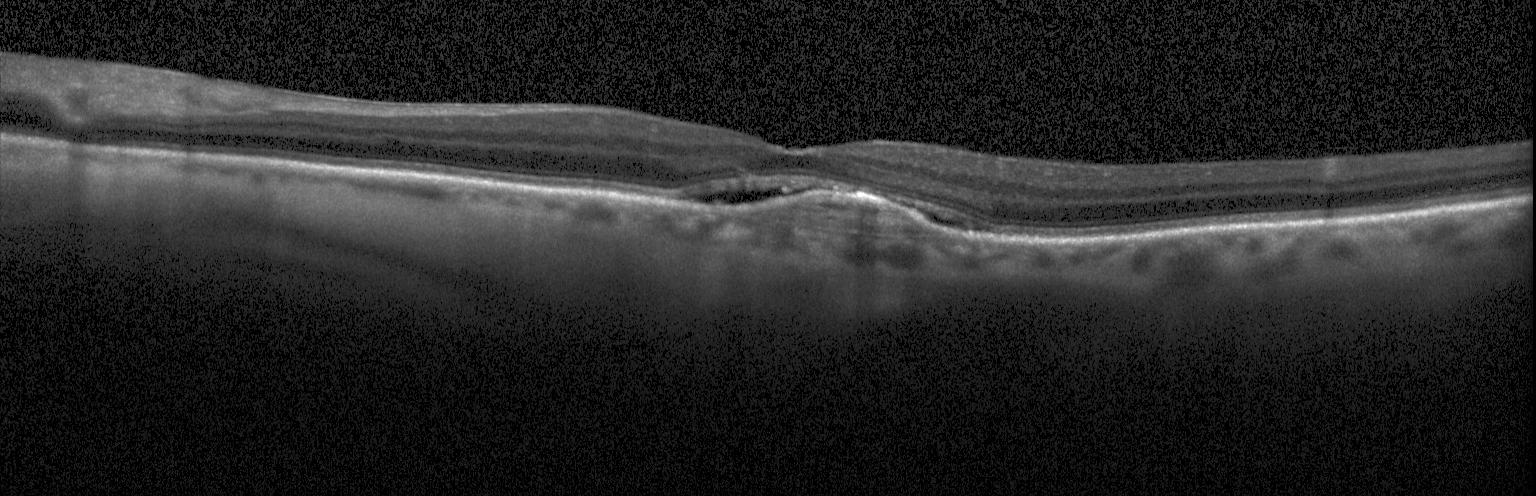

Diagnosis: a choroidal neovascular membrane.